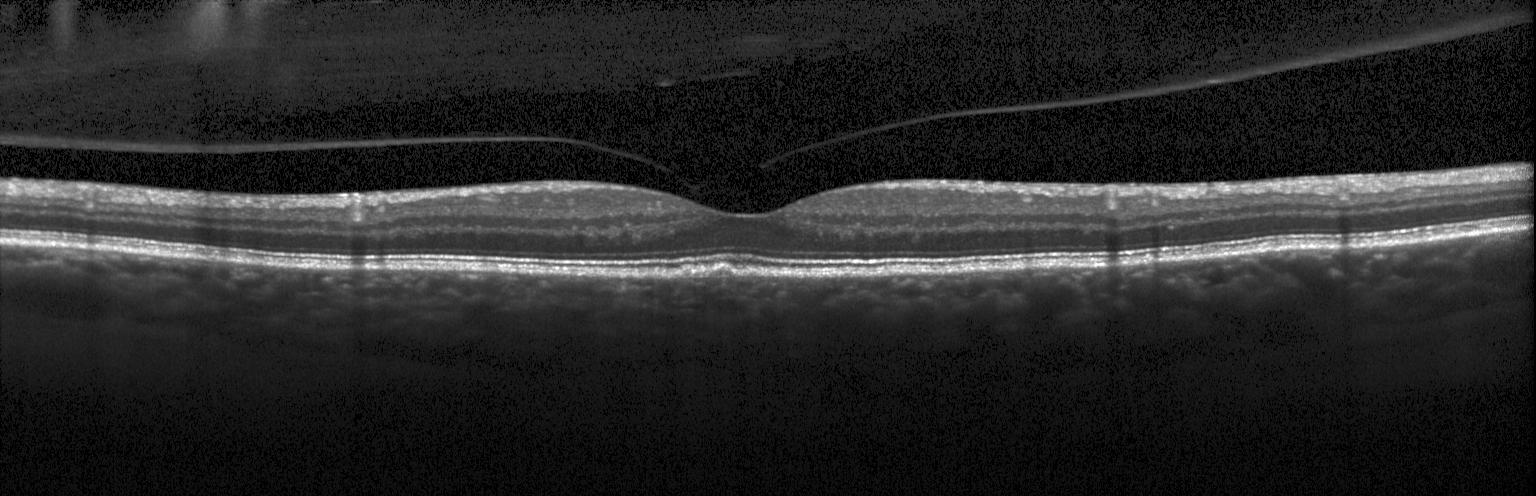

Sub-RPE drusenoid deposits.